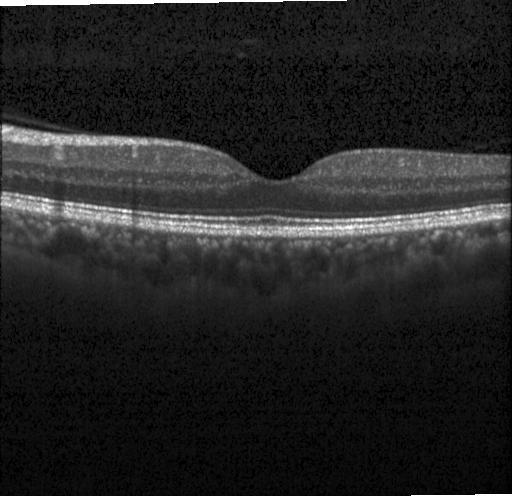

Spectral-domain optical coherence tomography; OCT line scan.
Diagnosis: no choroidal neovascularization, diabetic macular edema, or drusen.